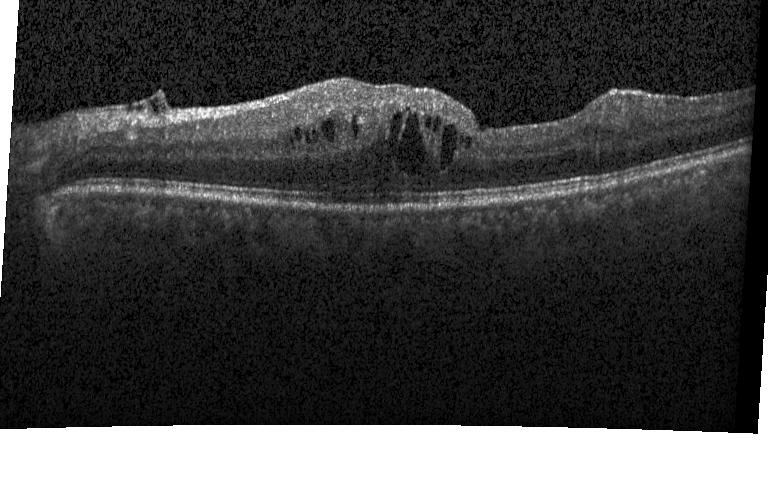

Diagnosis: diabetic macular edema (DME).